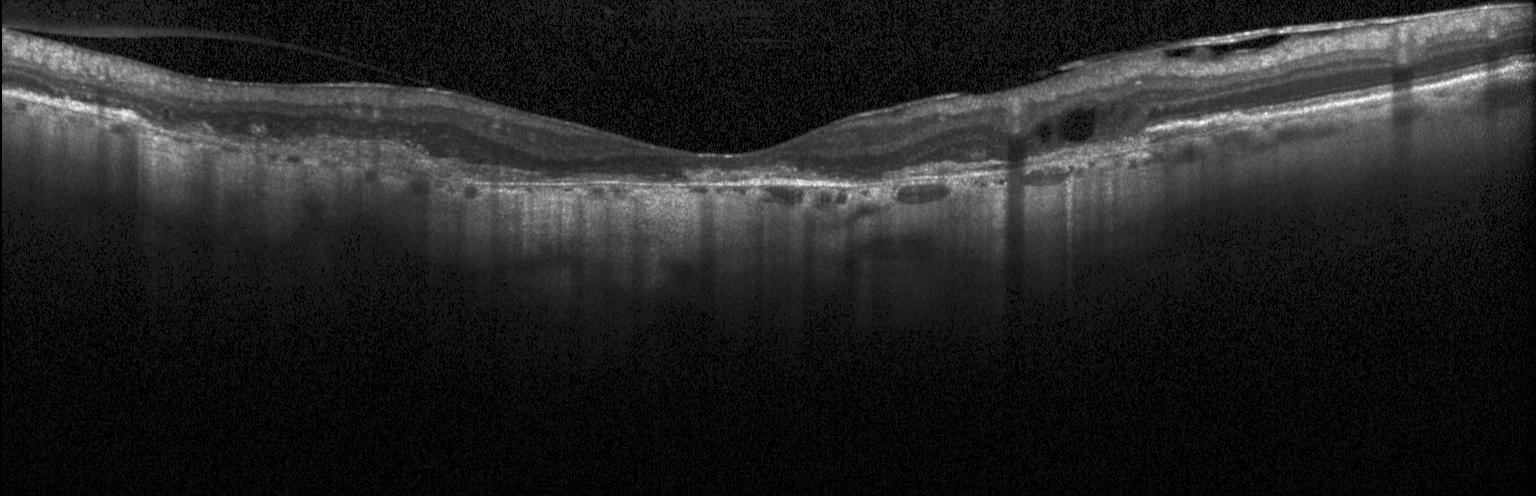 Horizontal scan through the fovea; instrument: Heidelberg Spectralis; spectral-domain optical coherence tomography; retinal OCT cross-section. Impression: a choroidal neovascular membrane.